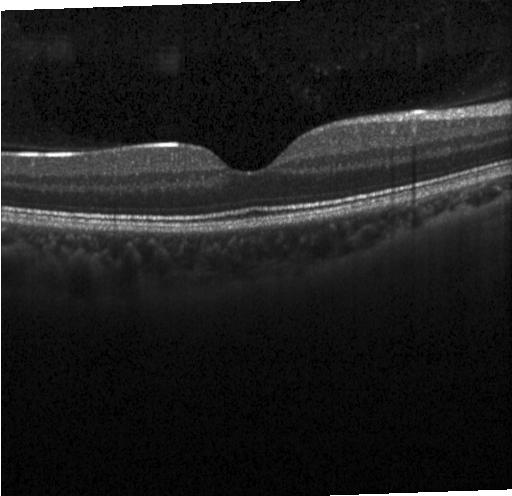 Heidelberg Spectralis, spectral-domain OCT, through the macula, retinal OCT B-scan.
Assessment: neither choroidal neovascularization, diabetic macular edema, nor drusen.